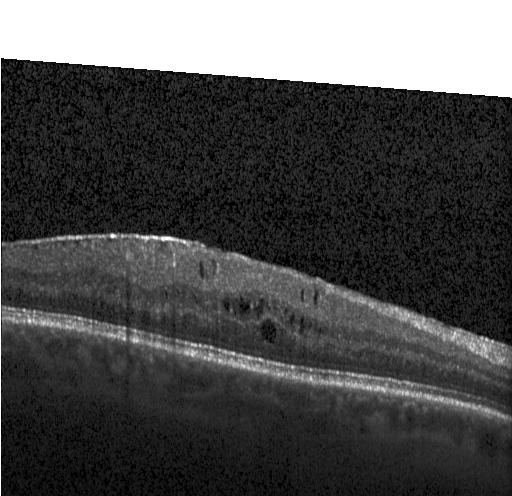

Spectral-domain OCT, Heidelberg Spectralis OCT system, optical coherence tomography B-scan.
Impression: diabetic macular edema.